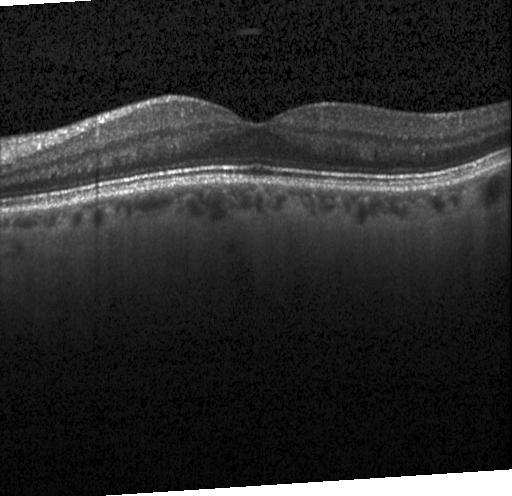
Retinal OCT B-scan.
Diagnosis: no evidence of choroidal neovascularization, diabetic macular edema, or drusen.